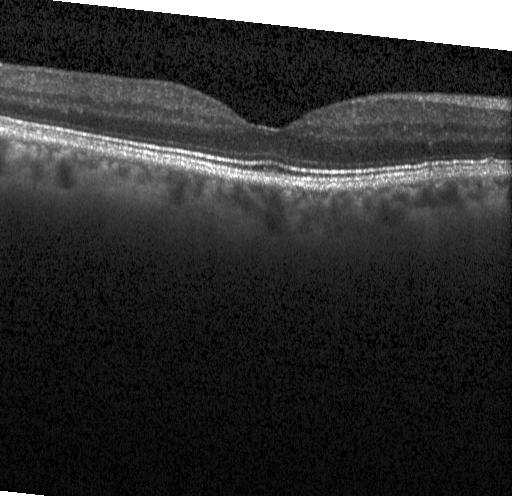 Finding: no evidence of CNV, DME, or drusen.